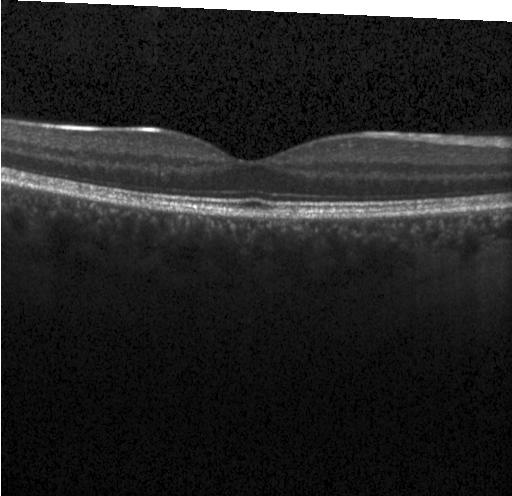

Horizontal scan through the fovea, spectral-domain OCT, optical coherence tomography scan. Diagnosis: no choroidal neovascularization, diabetic macular edema, or drusen.